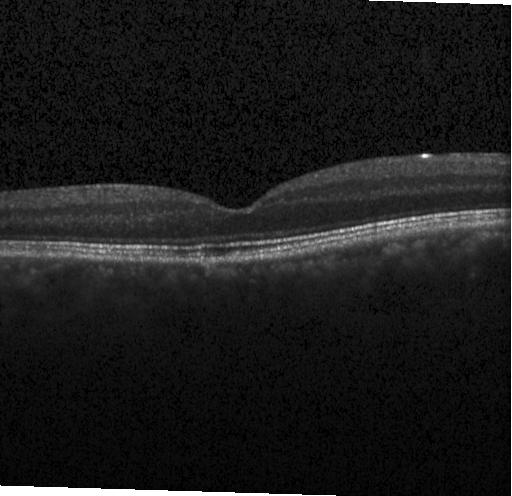 Fovea-centered · optical coherence tomography scan
This B-scan demonstrates neither choroidal neovascularization, diabetic macular edema, nor drusen.